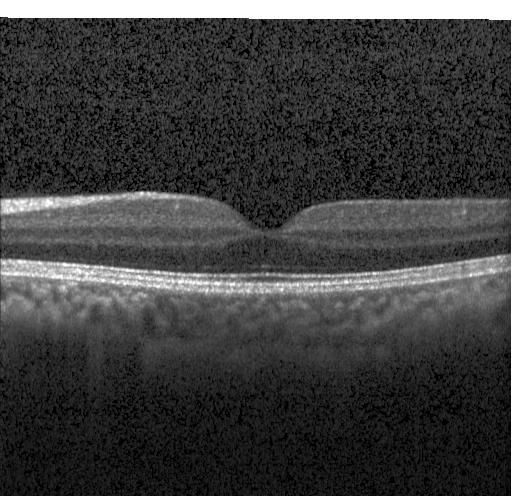
Retinal OCT B-scan. Dx: no choroidal neovascularization, no diabetic macular edema, and no drusen.